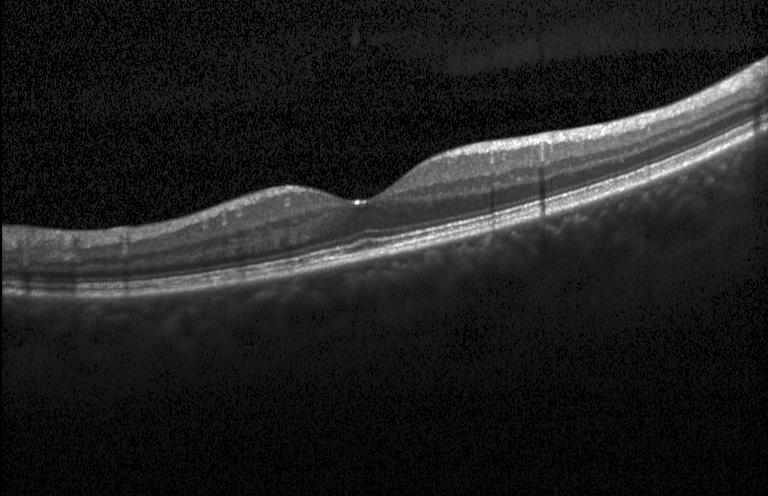

Spectral-domain OCT B-scan: neither choroidal neovascularization, diabetic macular edema, nor drusen.